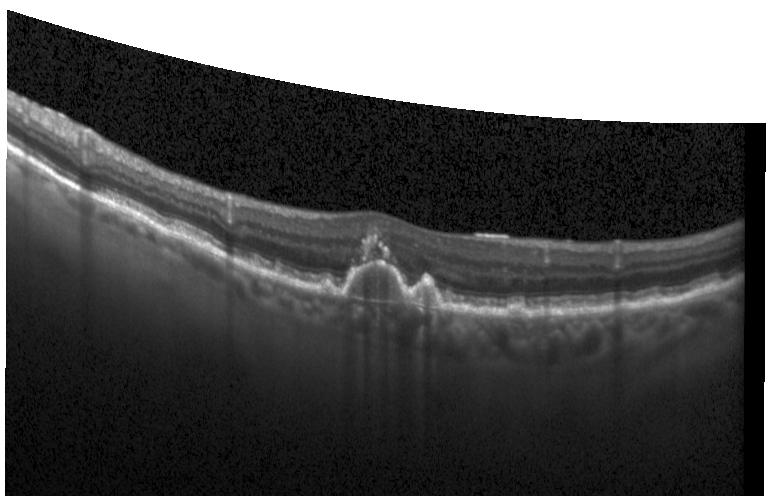

Instrument: Heidelberg Spectralis; fovea-centered; optical coherence tomography B-scan
Impression: a choroidal neovascular membrane.